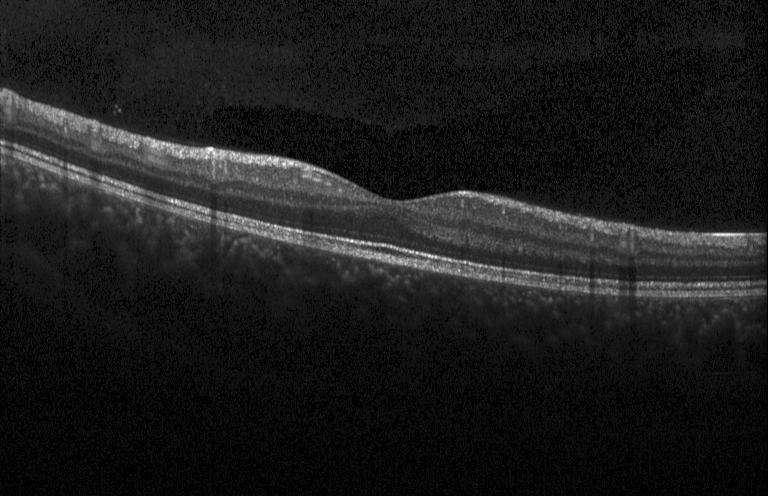

OCT B-scan showing no choroidal neovascularization, diabetic macular edema, or drusen.